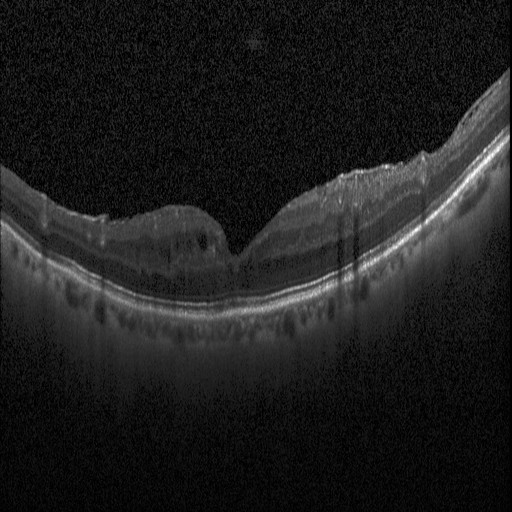
Instrument: Heidelberg Spectralis, retinal OCT cross-section, spectral-domain OCT. OCT finding: DME.